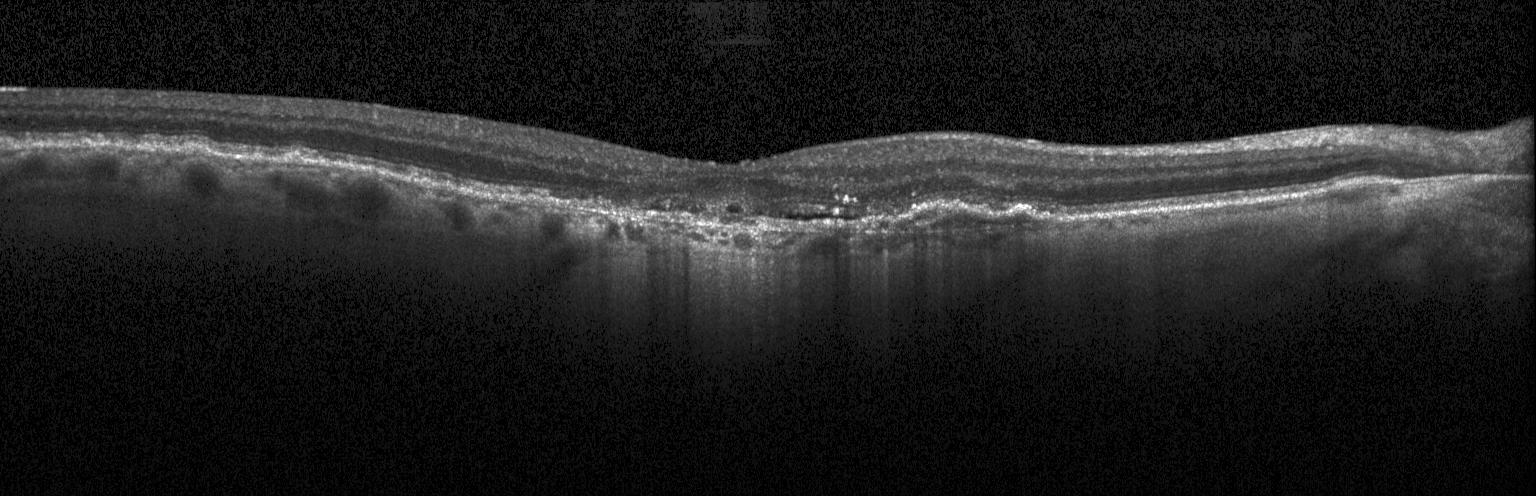

OCT B-scan showing a choroidal neovascular membrane.